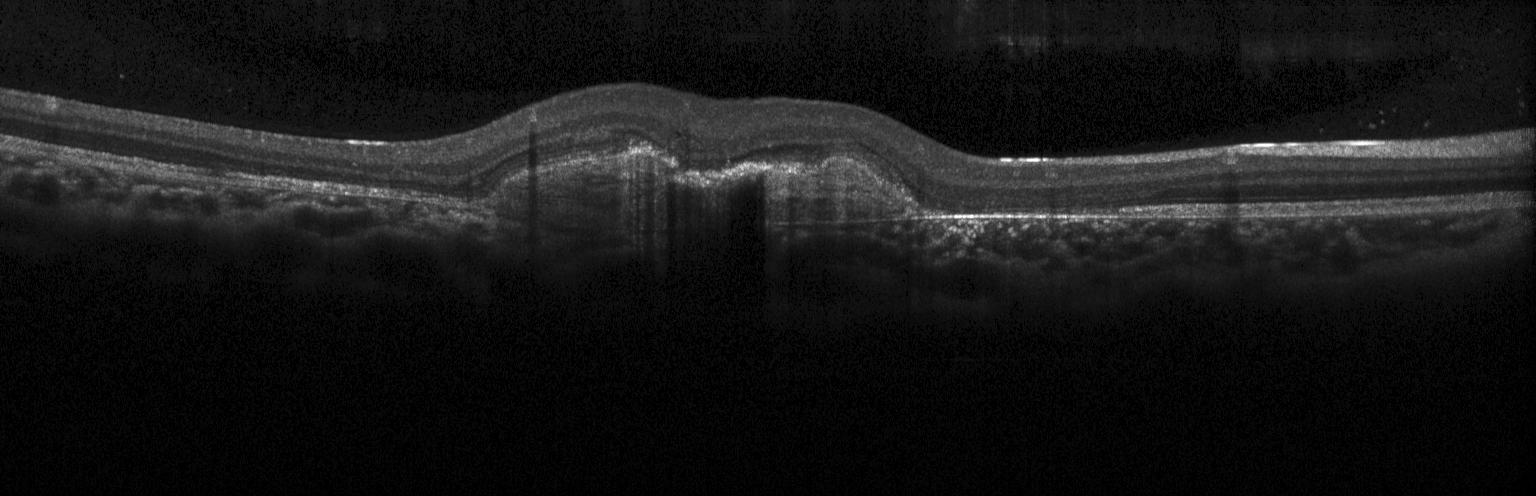

Optical coherence tomography scan, fovea-centered, Heidelberg Spectralis OCT system, spectral-domain optical coherence tomography.
The scan shows a choroidal neovascular membrane.